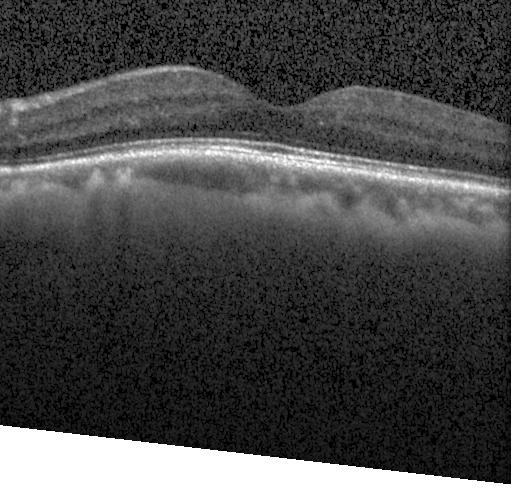

Optical coherence tomography scan
Impression: no choroidal neovascularization, no diabetic macular edema, and no drusen.